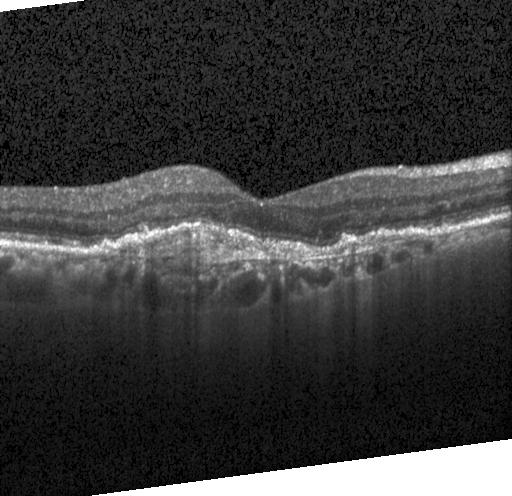 Horizontal scan through the fovea. OCT B-scan
The scan shows a choroidal neovascular membrane.